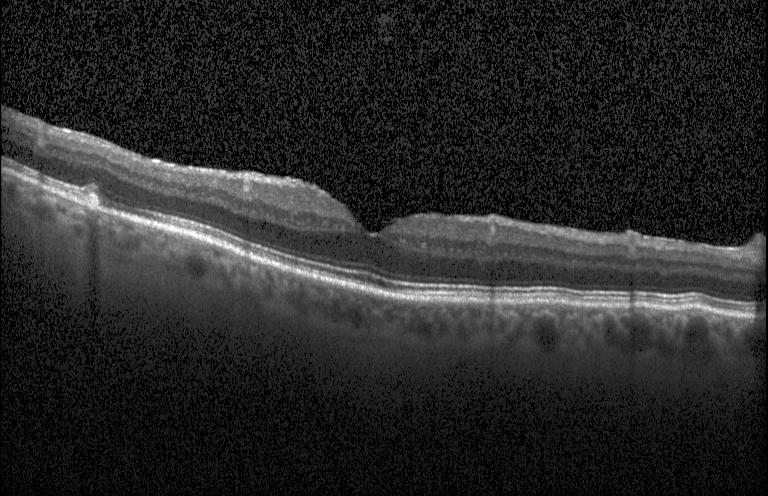 SD-OCT, acquired on a Heidelberg Spectralis, OCT line scan, through the macula
Diagnosis: sub-RPE drusenoid deposits.